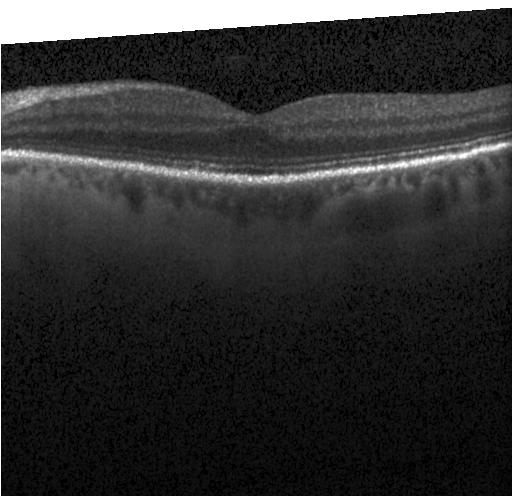
Spectral-domain OCT, acquired on a Heidelberg Spectralis, optical coherence tomography B-scan. Dx: neither choroidal neovascularization, diabetic macular edema, nor drusen.